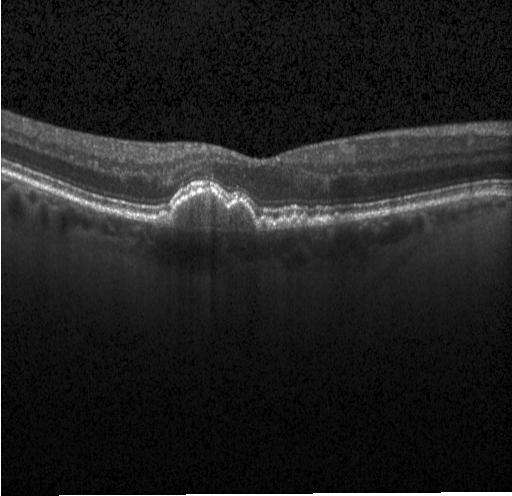 Optical coherence tomography B-scan — Diagnosis: a choroidal neovascular membrane.